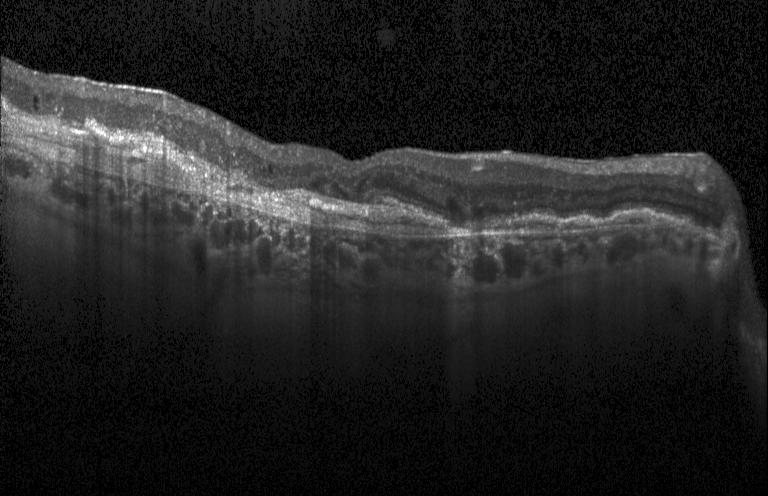 Finding: CNV.